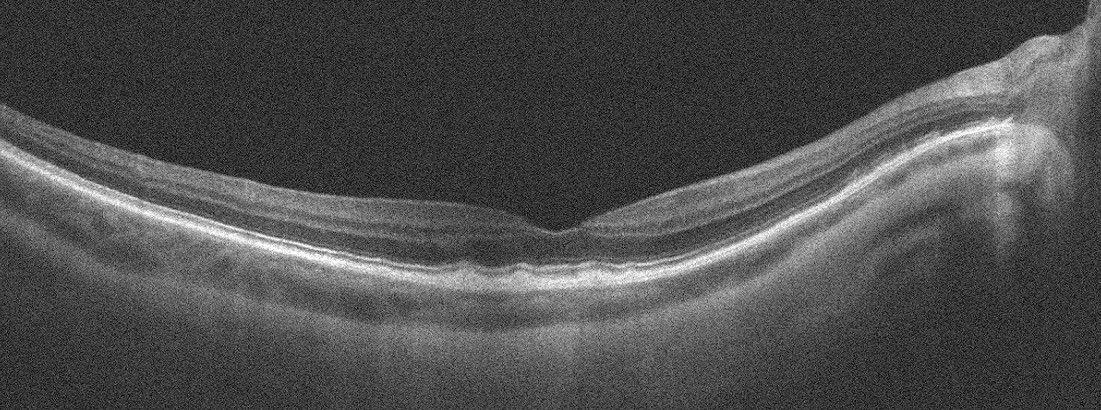

Fovea-centered; optical coherence tomography scan. This B-scan demonstrates age-related macular degeneration (AMD).